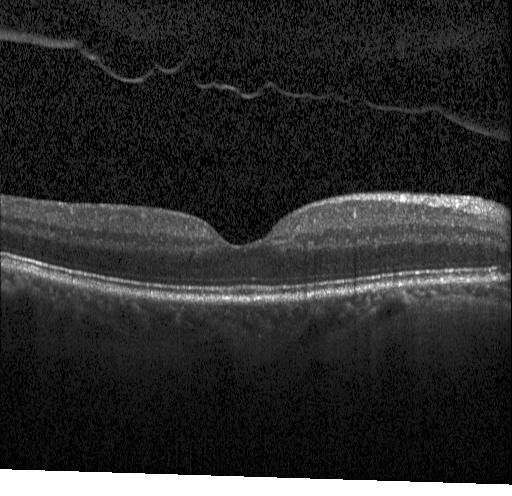 OCT B-scan — The scan shows neither choroidal neovascularization, diabetic macular edema, nor drusen.